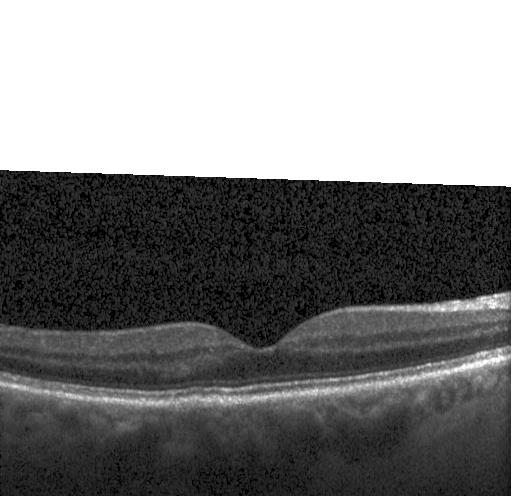 This B-scan demonstrates neither choroidal neovascularization, diabetic macular edema, nor drusen.